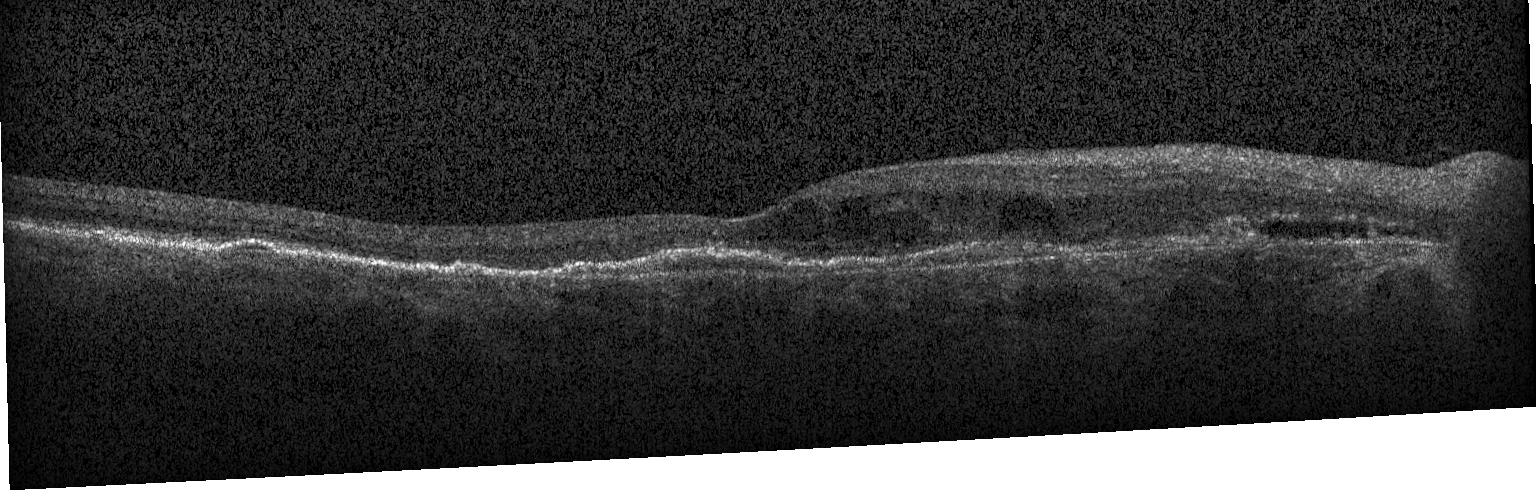 Spectral-domain OCT; OCT line scan
Finding: a choroidal neovascular membrane.